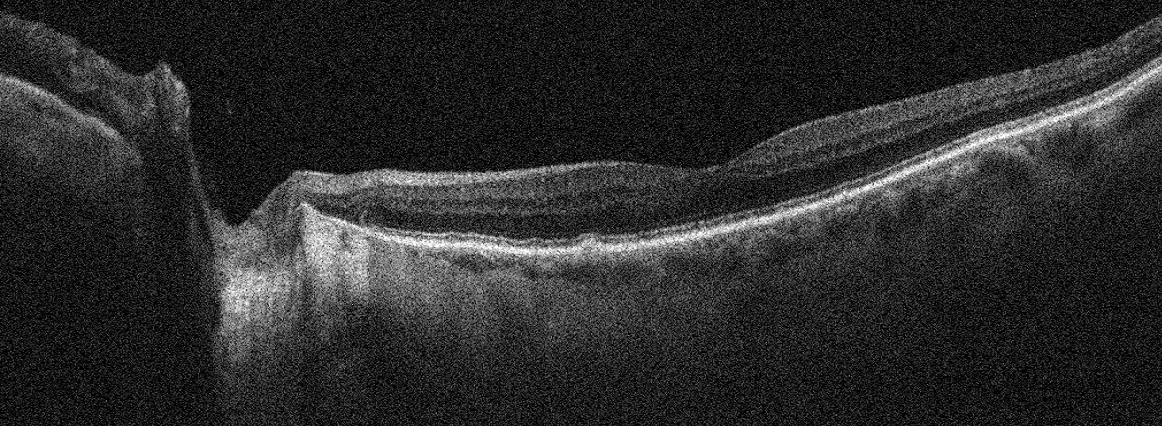
Oculus sinister · optical coherence tomography scan · instrument: Optovue Avanti RTVue XR.
This B-scan demonstrates age-related macular degeneration.